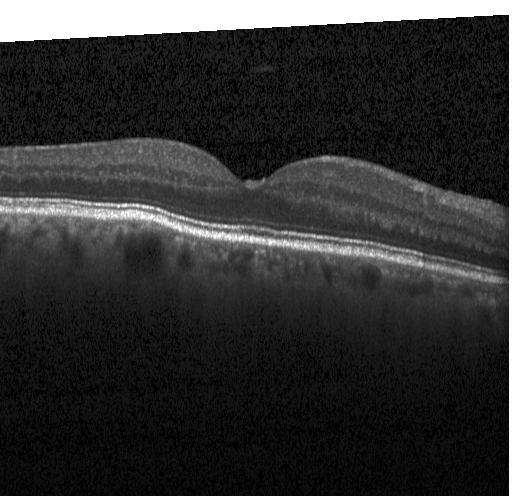 Macular OCT: no choroidal neovascularization, diabetic macular edema, or drusen.